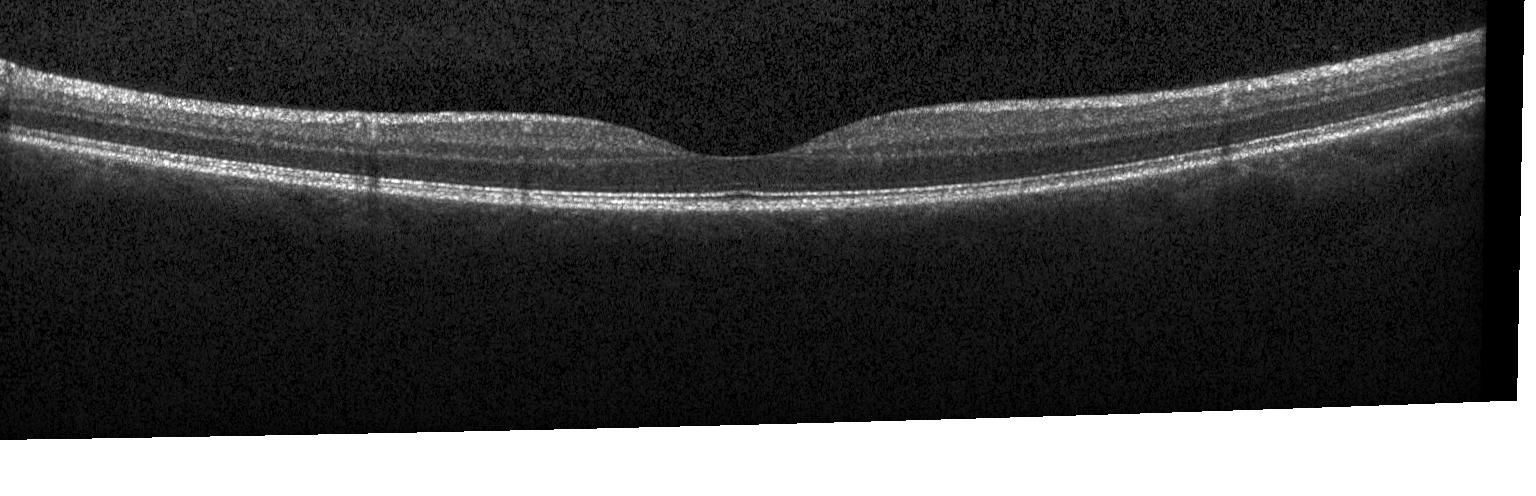
OCT B-scan; spectral-domain OCT.
Macular OCT: no evidence of CNV, DME, or drusen.